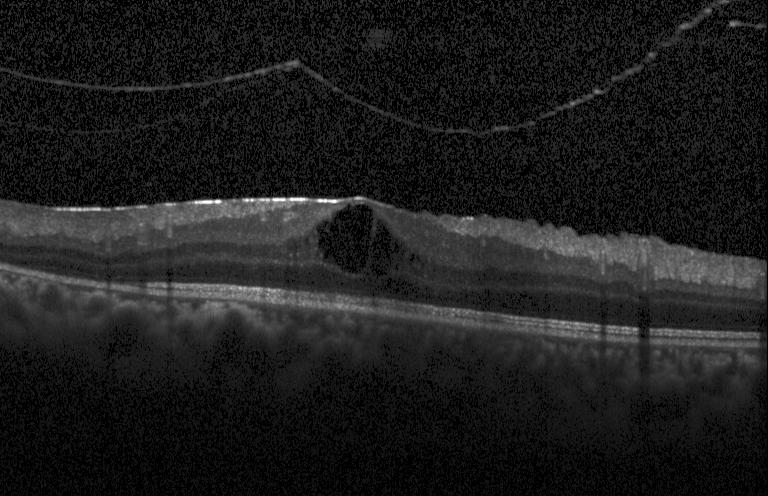 Retinal OCT B-scan · fovea-centered. Impression: diabetic macular edema (DME).